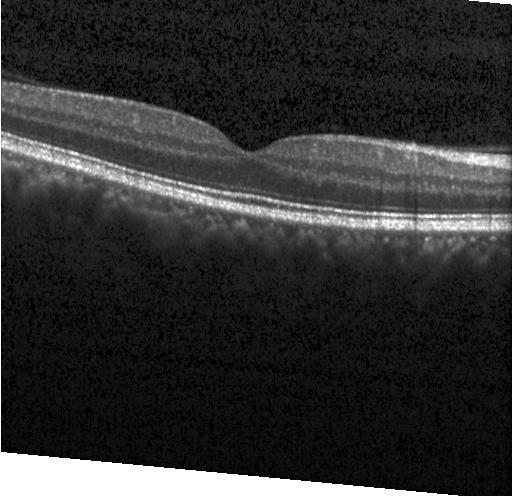 SD-OCT · instrument: Heidelberg Spectralis · OCT line scan.
Diagnosis: no evidence of choroidal neovascularization, diabetic macular edema, or drusen.